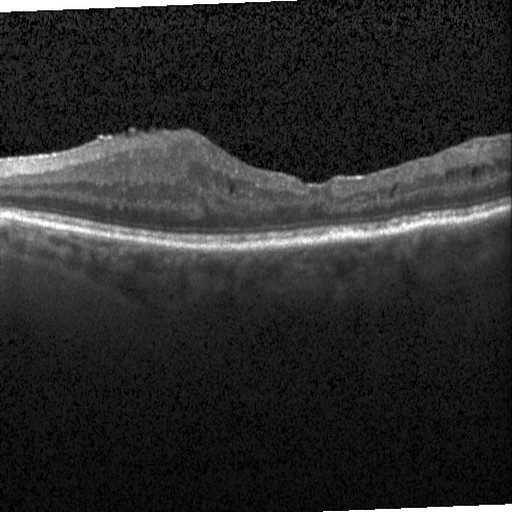
Centered on the fovea · Heidelberg Spectralis · OCT B-scan · spectral-domain OCT
Diagnosis: diabetic macular edema (DME).